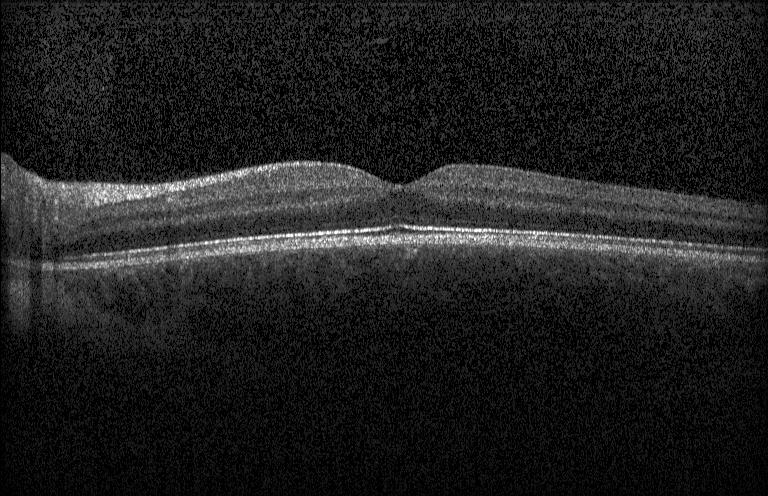
Finding: no choroidal neovascularization, no diabetic macular edema, and no drusen.